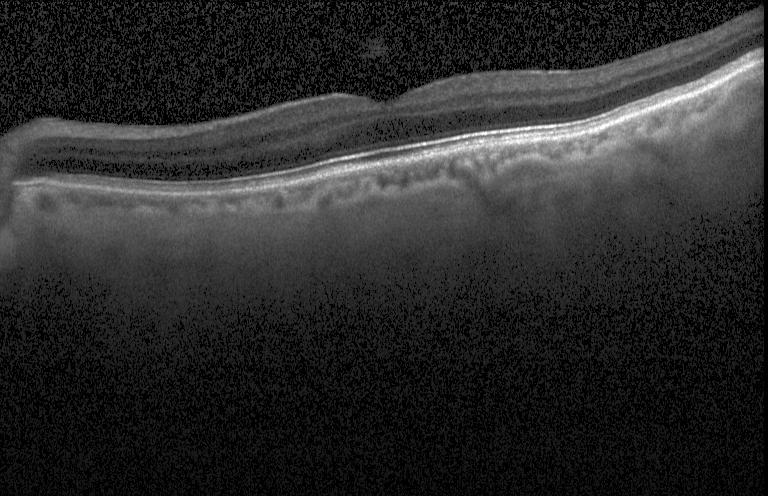 Retinal OCT B-scan · through the macula · Heidelberg Spectralis OCT system. The scan shows no choroidal neovascularization, no diabetic macular edema, and no drusen.